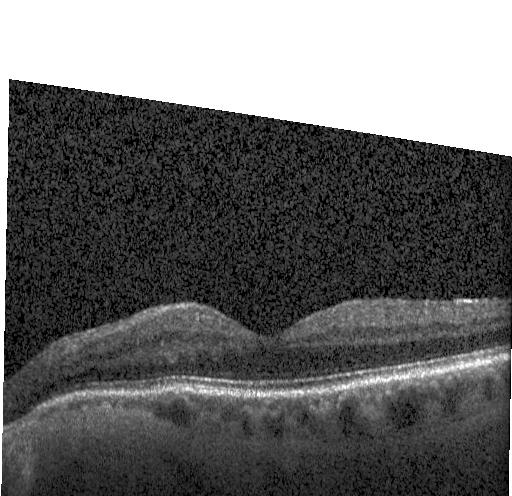 Retinal OCT cross-section — Impression: no evidence of CNV, DME, or drusen.